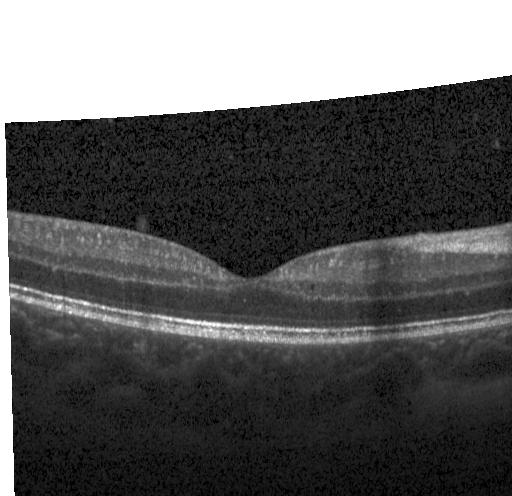

Macular scan; retinal OCT cross-section.
Diagnosis: no evidence of CNV, DME, or drusen.